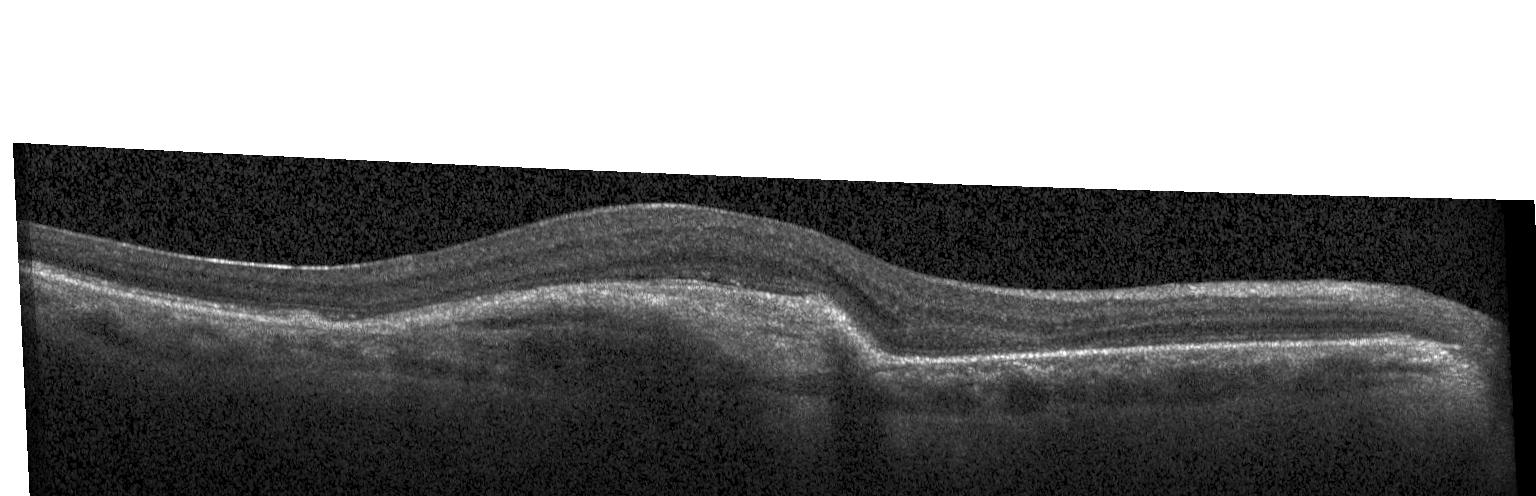
Optical coherence tomography B-scan; SD-OCT; Heidelberg Spectralis; fovea-centered.
Impression: choroidal neovascularization (CNV).